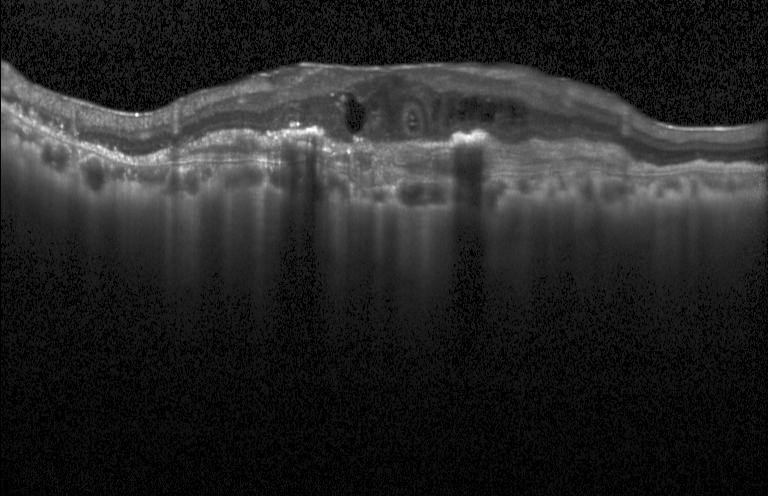

Retinal OCT cross-section · fovea-centered · SD-OCT · Heidelberg Spectralis.
Impression: choroidal neovascularization (CNV).